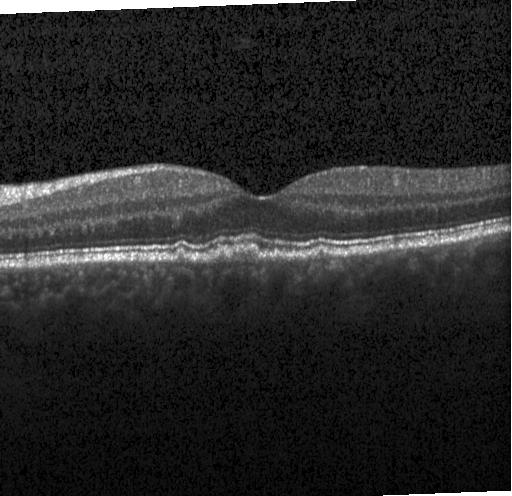

Dx: drusen.